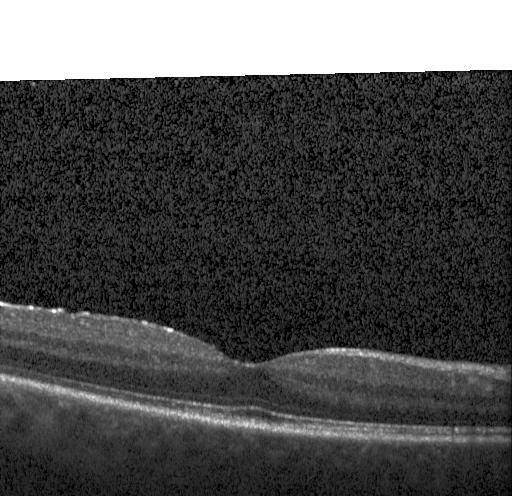
Spectral-domain OCT · optical coherence tomography scan · acquired on a Heidelberg Spectralis — OCT finding: no choroidal neovascularization, diabetic macular edema, or drusen.